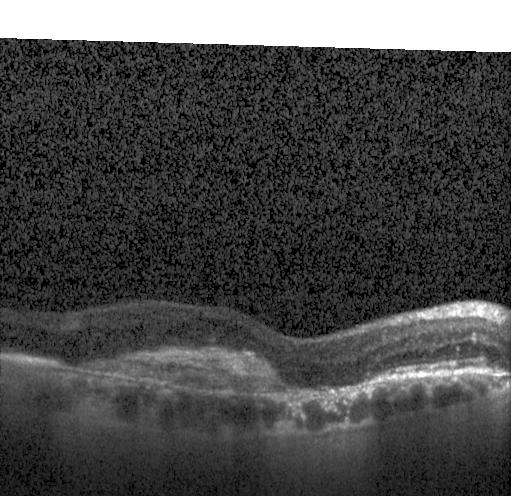

Finding: a choroidal neovascular membrane.